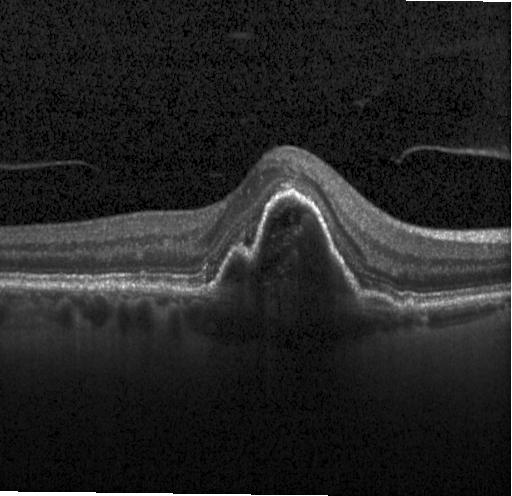 Retinal OCT cross-section; acquired on a Heidelberg Spectralis; through the macula; SD-OCT.
Finding: CNV.